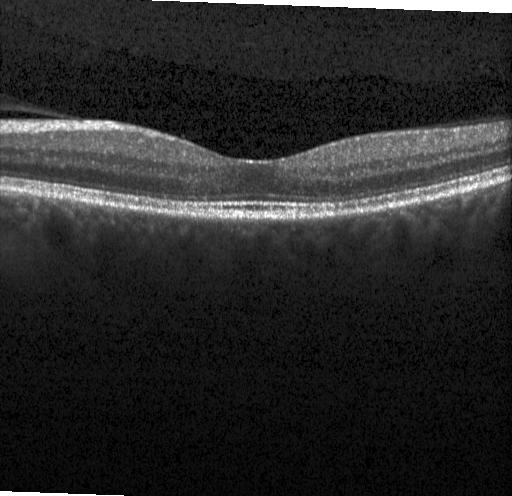
This B-scan demonstrates neither choroidal neovascularization, diabetic macular edema, nor drusen.